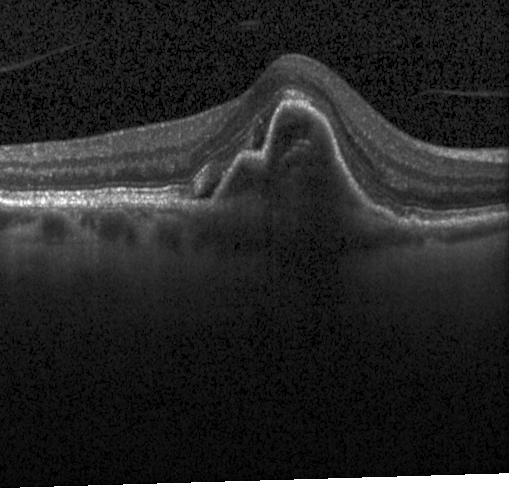

OCT finding: a choroidal neovascular membrane.